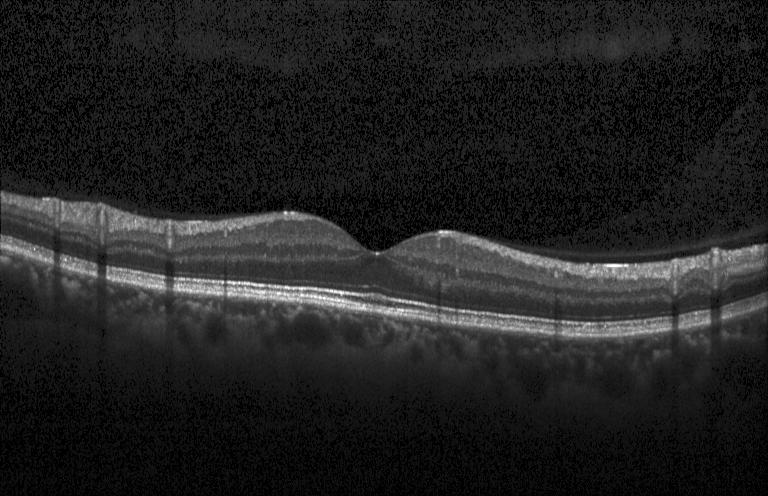 Spectral-domain OCT, OCT line scan, horizontal scan through the fovea.
Dx: neither choroidal neovascularization, diabetic macular edema, nor drusen.